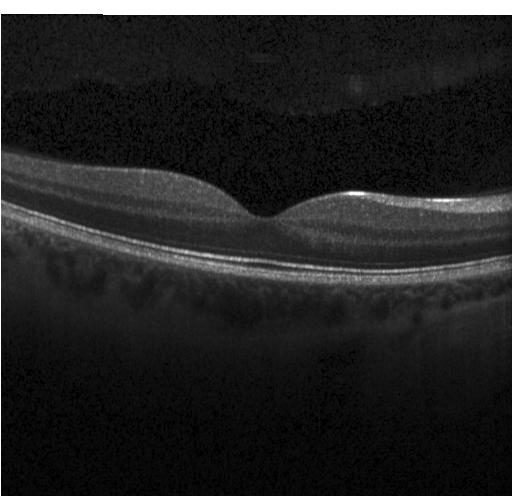

Optical coherence tomography B-scan — Diagnosis: neither choroidal neovascularization, diabetic macular edema, nor drusen.